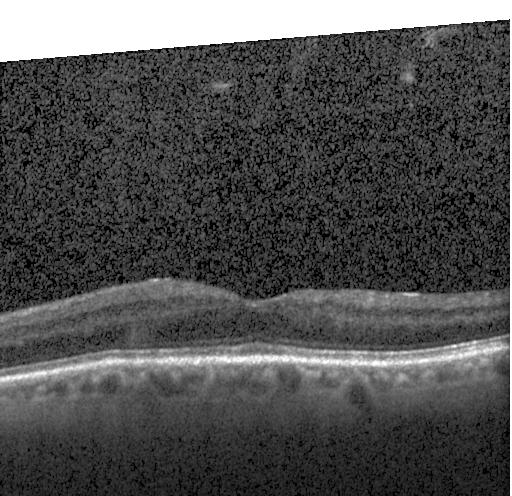 Macular scan, instrument: Heidelberg Spectralis, optical coherence tomography B-scan
Impression: no CNV, DME, or drusen.